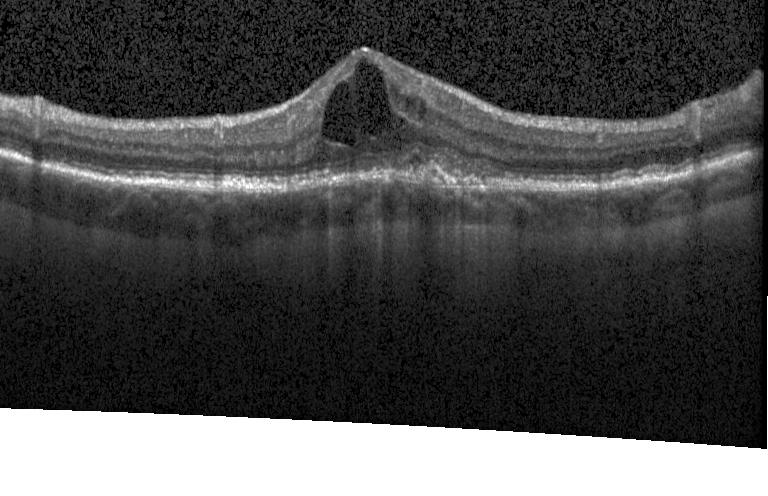
Heidelberg Spectralis, centered on the fovea, retinal OCT B-scan — Assessment: choroidal neovascularization.